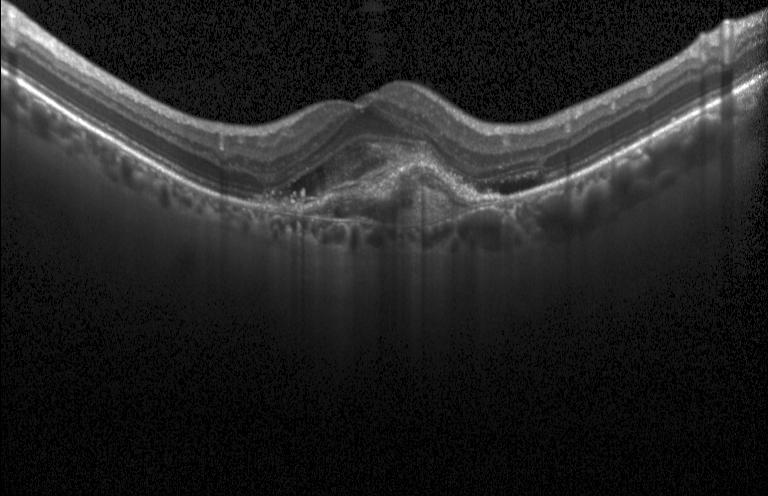

OCT B-scan
This B-scan demonstrates CNV.